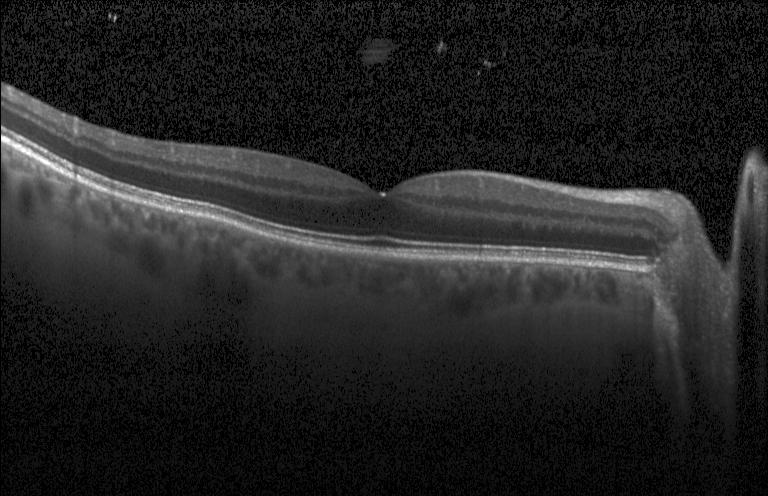
Spectral-domain optical coherence tomography. Macular scan. Retinal OCT cross-section. Macular OCT: neither choroidal neovascularization, diabetic macular edema, nor drusen.